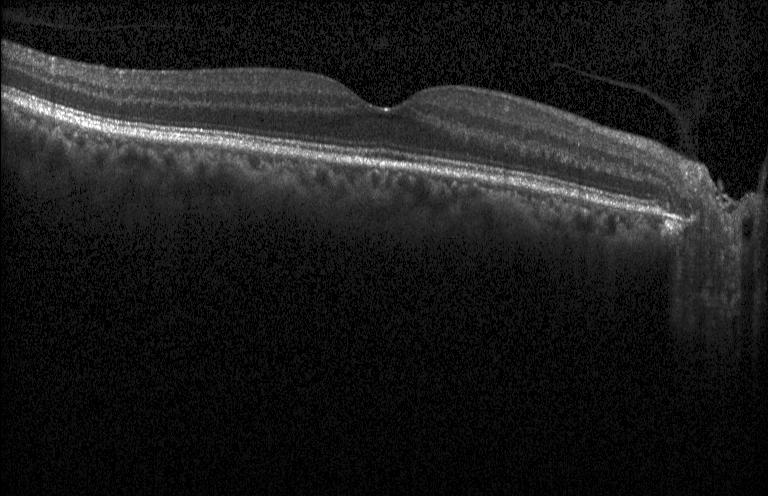

Macular OCT demonstrating neither choroidal neovascularization, diabetic macular edema, nor drusen.